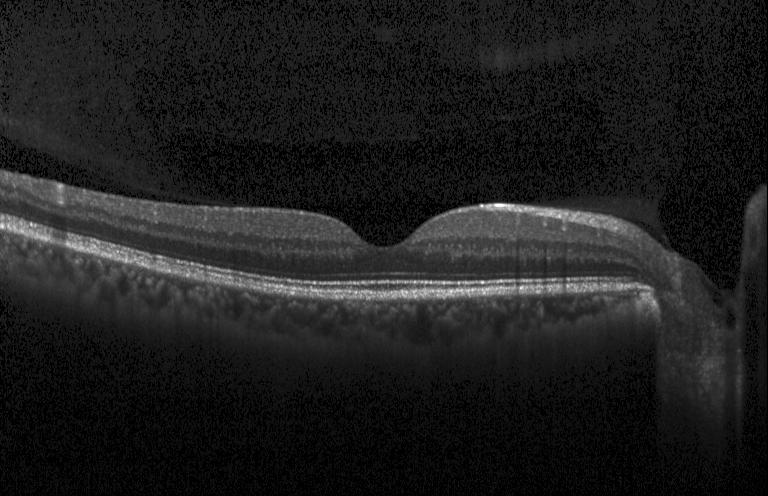

Macular OCT demonstrating no evidence of CNV, DME, or drusen.